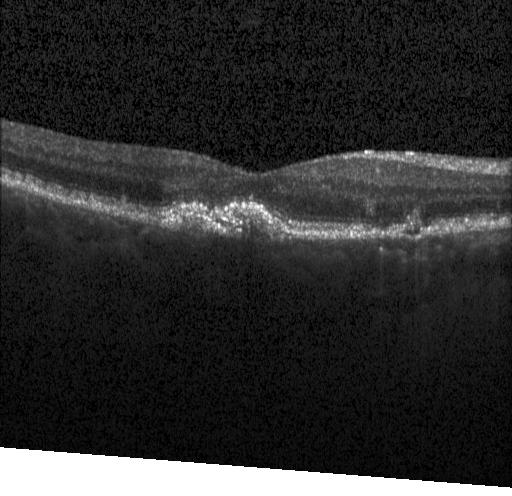
Retinal OCT B-scan. A choroidal neovascular membrane.